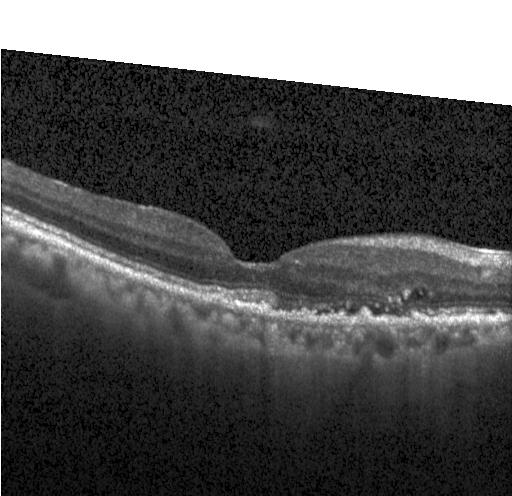 This B-scan demonstrates a choroidal neovascular membrane.